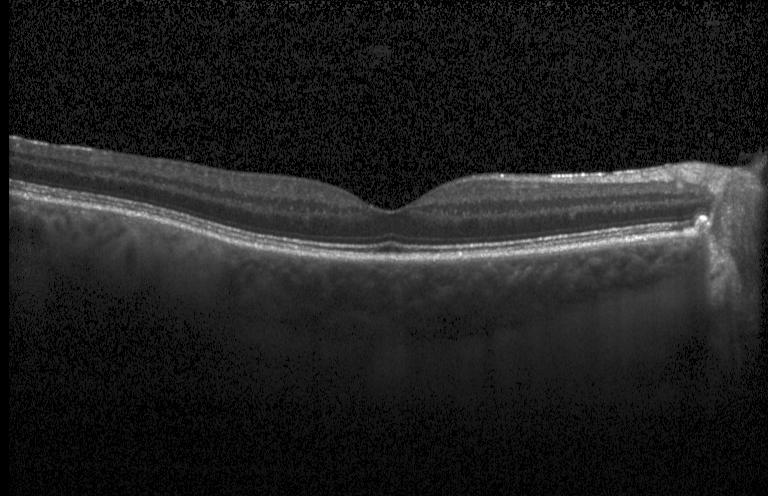
Diagnosis: no choroidal neovascularization, no diabetic macular edema, and no drusen.